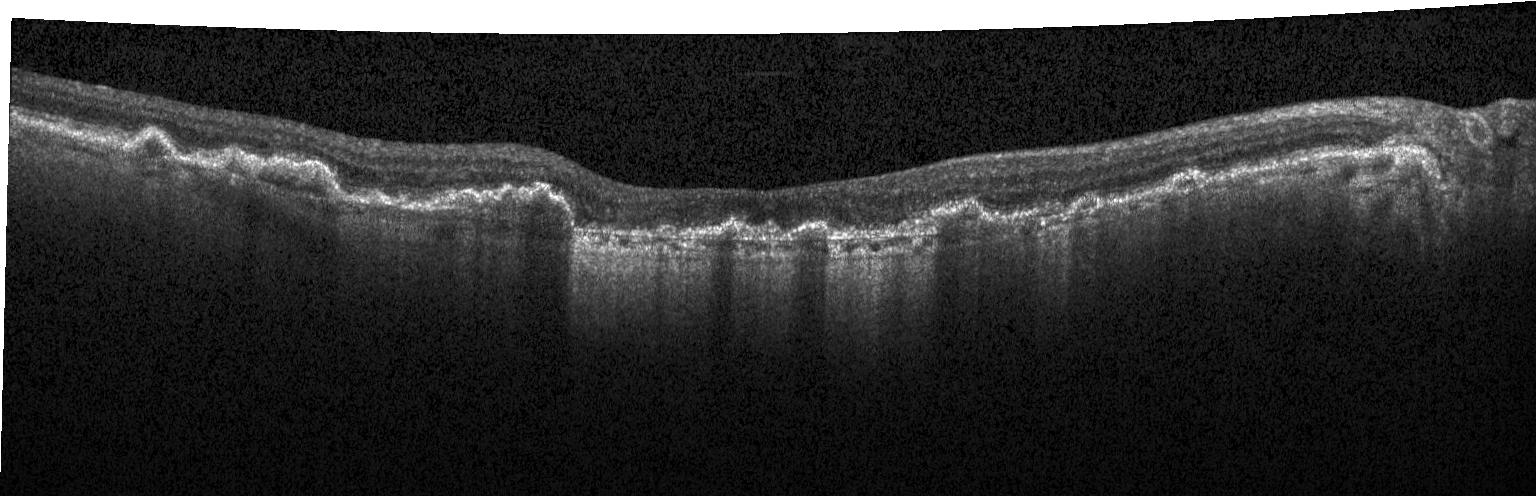
Optical coherence tomography scan; SD-OCT; horizontal scan through the fovea.
Finding: choroidal neovascularization.